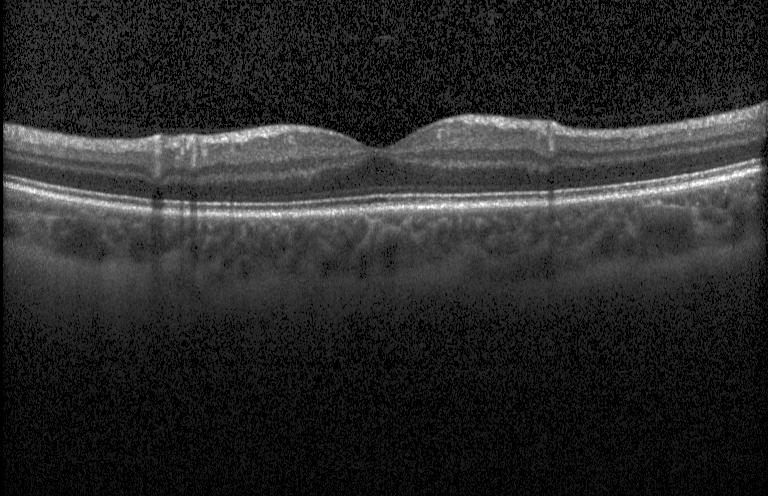
Horizontal scan through the fovea, OCT line scan, Heidelberg Spectralis. Dx: no choroidal neovascularization, diabetic macular edema, or drusen.